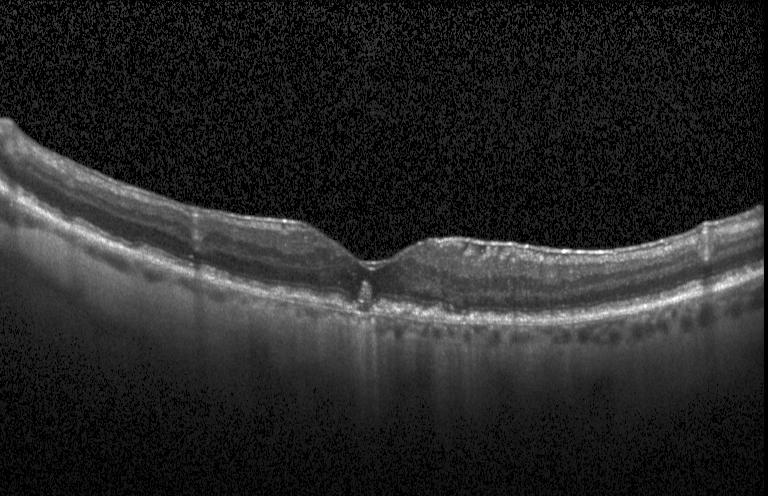
OCT line scan
Finding: multiple drusen.